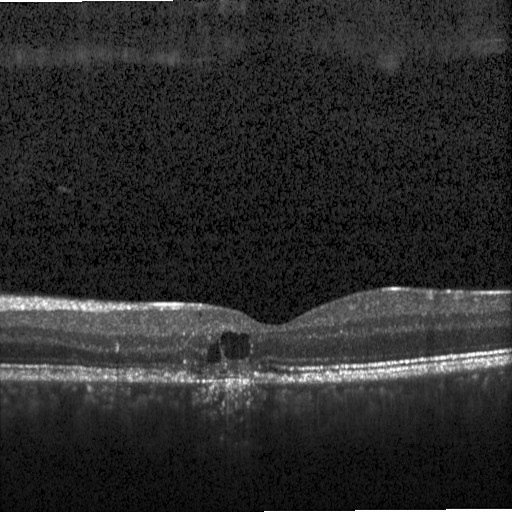

Macular scan, spectral-domain OCT, optical coherence tomography B-scan. Dx: DME.